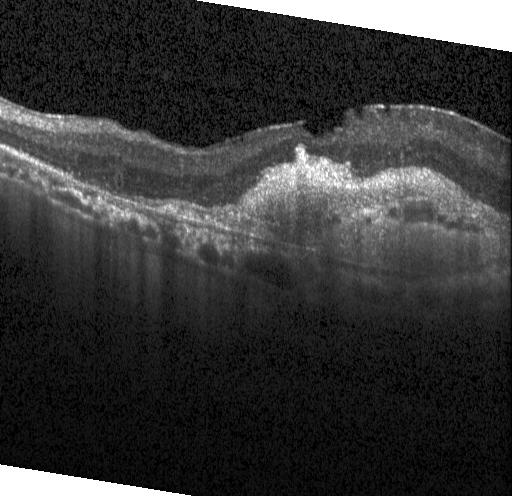

Assessment: CNV.